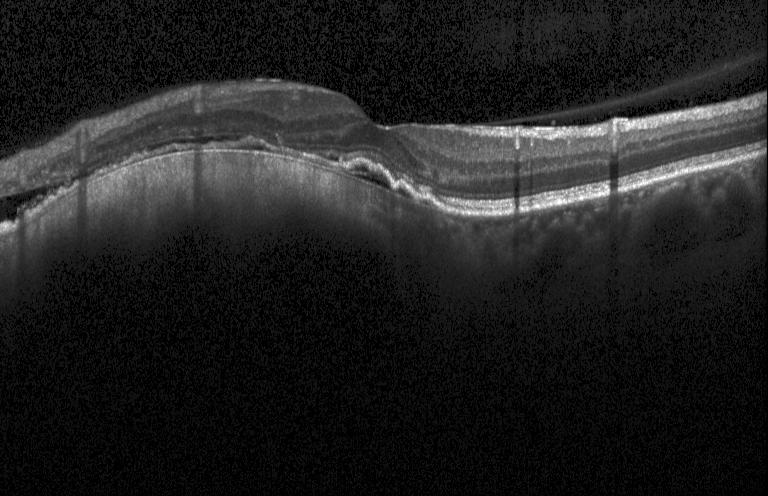
Acquired on a Heidelberg Spectralis. Spectral-domain OCT. OCT B-scan. Horizontal scan through the fovea — Finding: choroidal neovascularization (CNV).